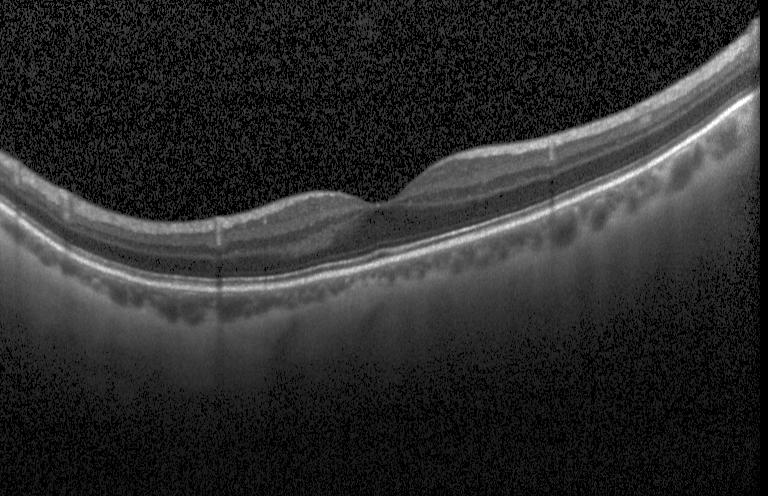
Heidelberg Spectralis OCT system. Centered on the fovea. OCT B-scan.
Impression: neither choroidal neovascularization, diabetic macular edema, nor drusen.